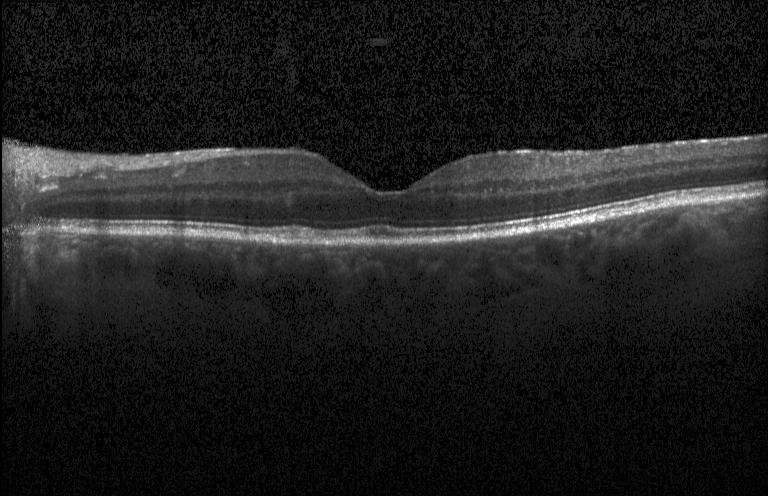 Acquired on a Heidelberg Spectralis; horizontal scan through the fovea; SD-OCT; retinal OCT cross-section — Finding: neither choroidal neovascularization, diabetic macular edema, nor drusen.